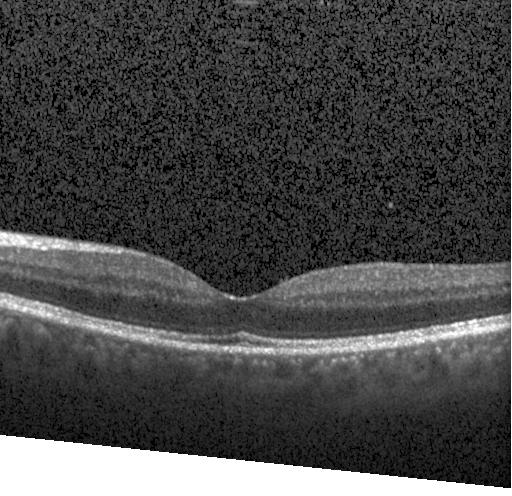 OCT finding: neither choroidal neovascularization, diabetic macular edema, nor drusen.